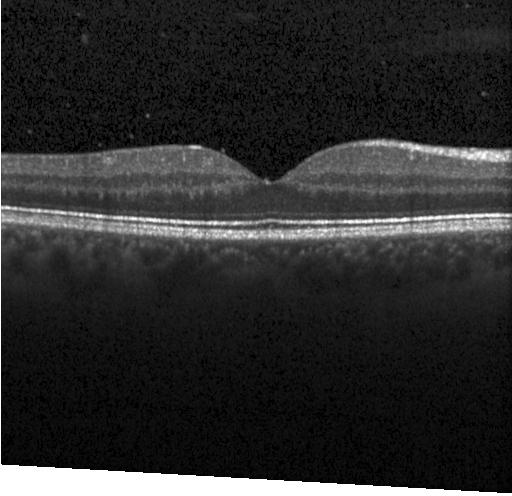

Macular OCT: no evidence of choroidal neovascularization, diabetic macular edema, or drusen.